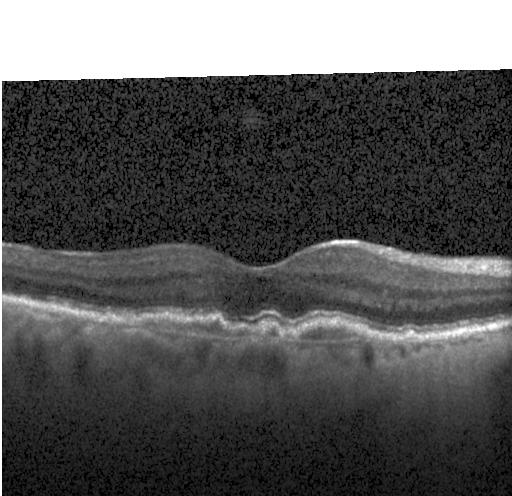
OCT line scan, Heidelberg Spectralis — Finding: a choroidal neovascular membrane.